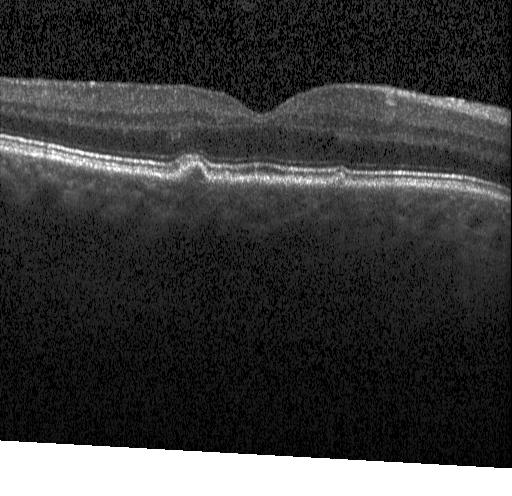 Retinal OCT cross-section showing drusen.